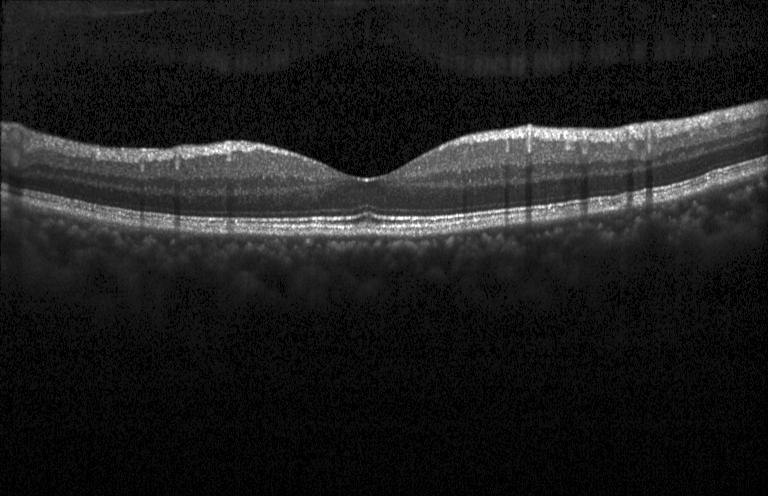 Macular OCT demonstrating no choroidal neovascularization, no diabetic macular edema, and no drusen.